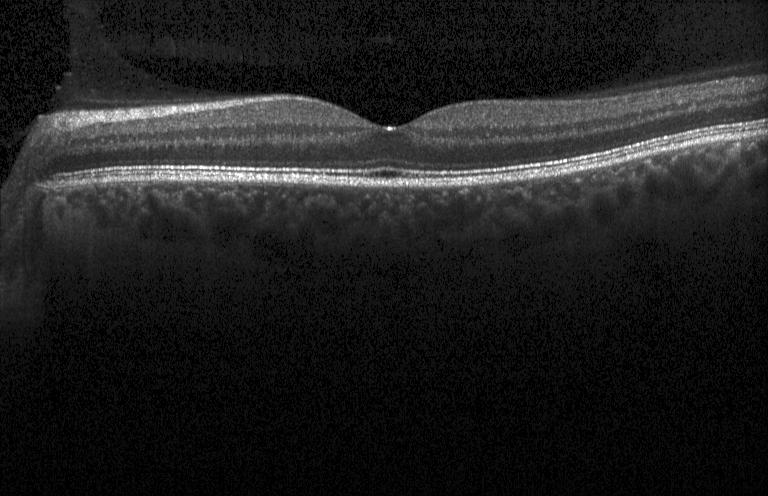
Impression: neither choroidal neovascularization, diabetic macular edema, nor drusen.